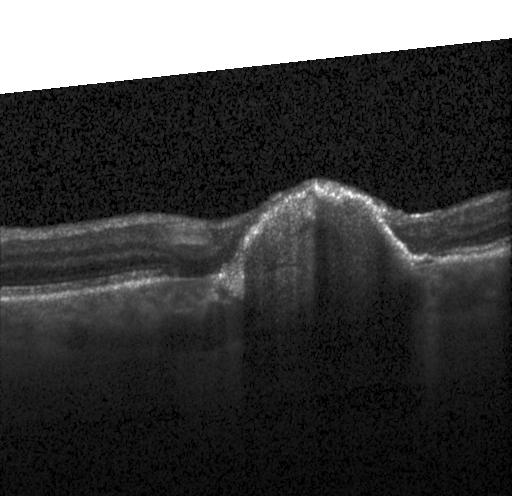

Dx: CNV.